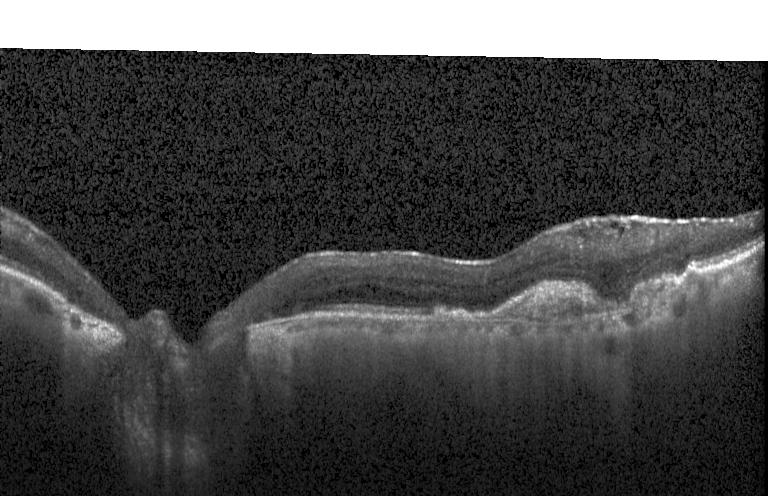
Impression: choroidal neovascularization (CNV).